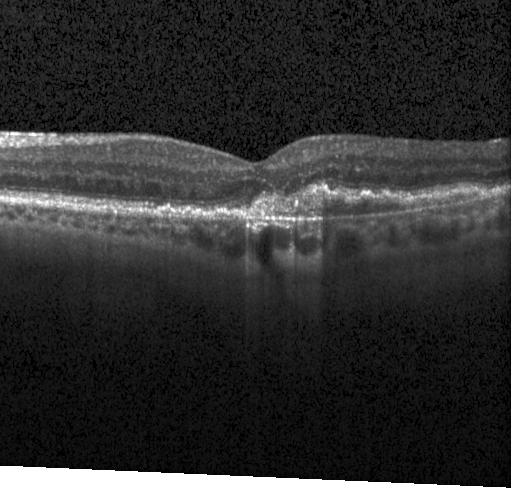

Centered on the fovea · optical coherence tomography scan · instrument: Heidelberg Spectralis · SD-OCT — Dx: choroidal neovascularization.